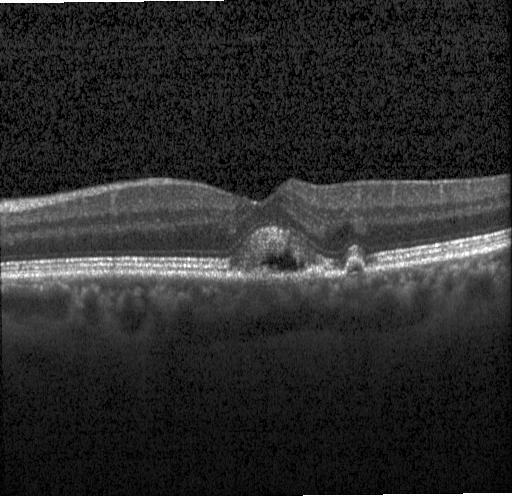
Assessment: CNV.